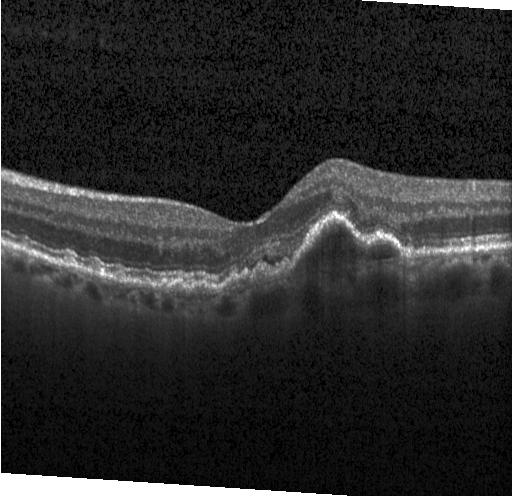 Horizontal scan through the fovea · acquired on a Heidelberg Spectralis · spectral-domain optical coherence tomography · OCT B-scan — Assessment: a choroidal neovascular membrane.